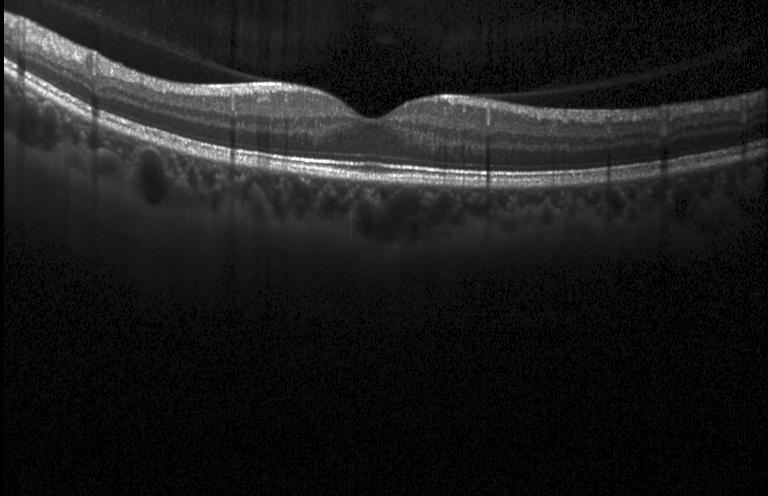 OCT B-scan. Heidelberg Spectralis
Diagnosis: no evidence of CNV, DME, or drusen.